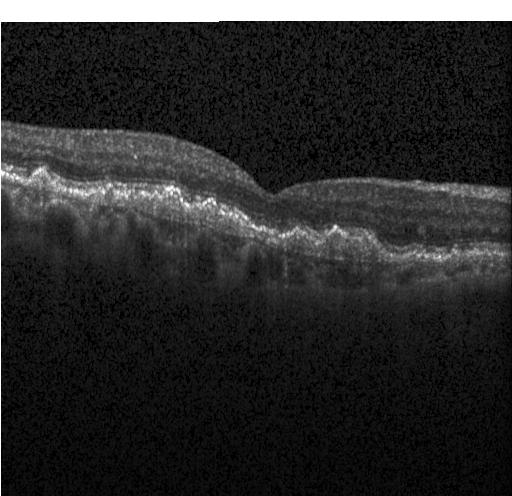
Spectral-domain OCT B-scan: CNV.